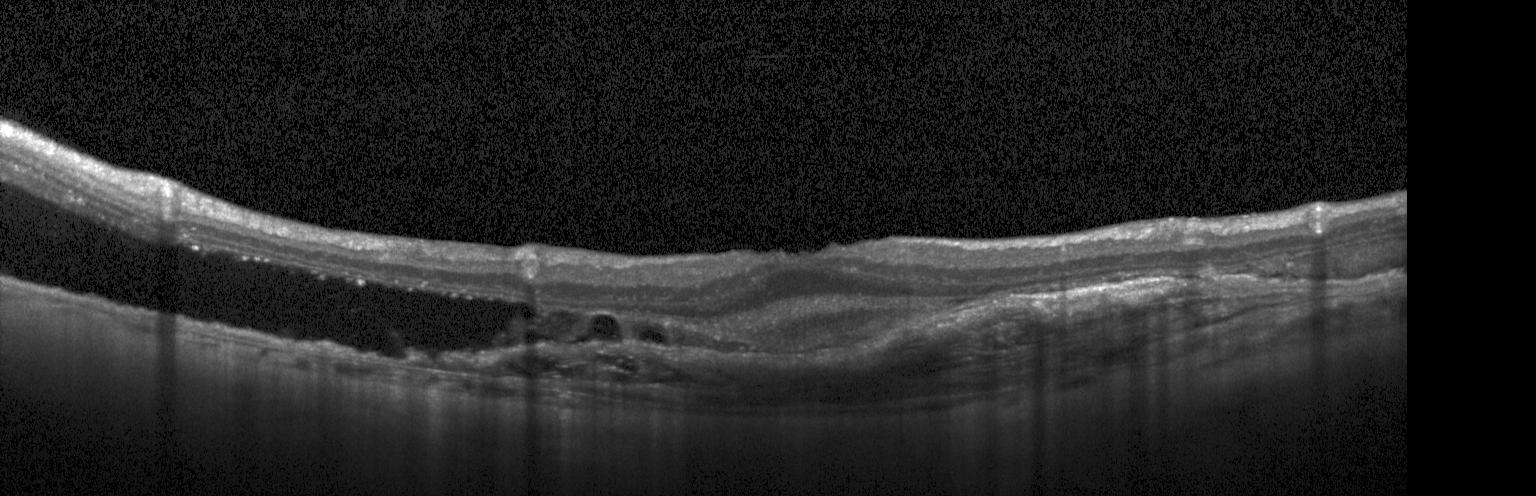

Finding: choroidal neovascularization.